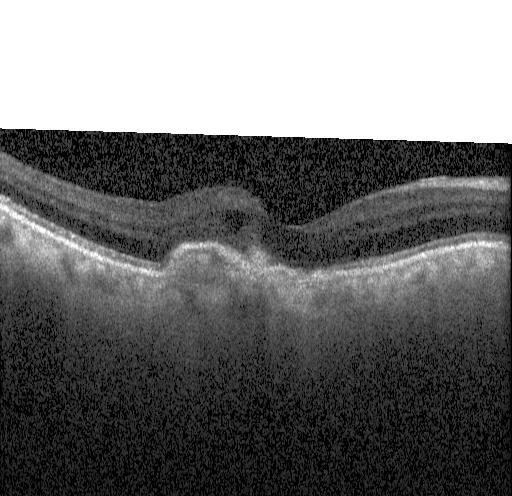
Retinal OCT cross-section. Instrument: Heidelberg Spectralis. Dx: choroidal neovascularization.